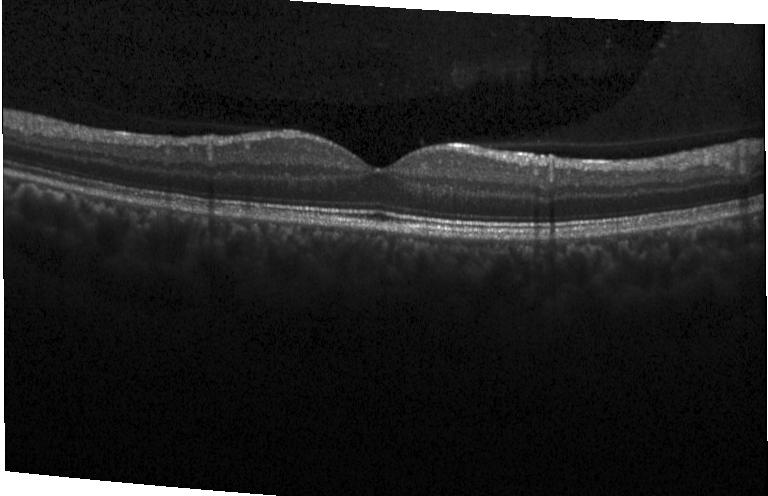
Macular OCT: no choroidal neovascularization, no diabetic macular edema, and no drusen.